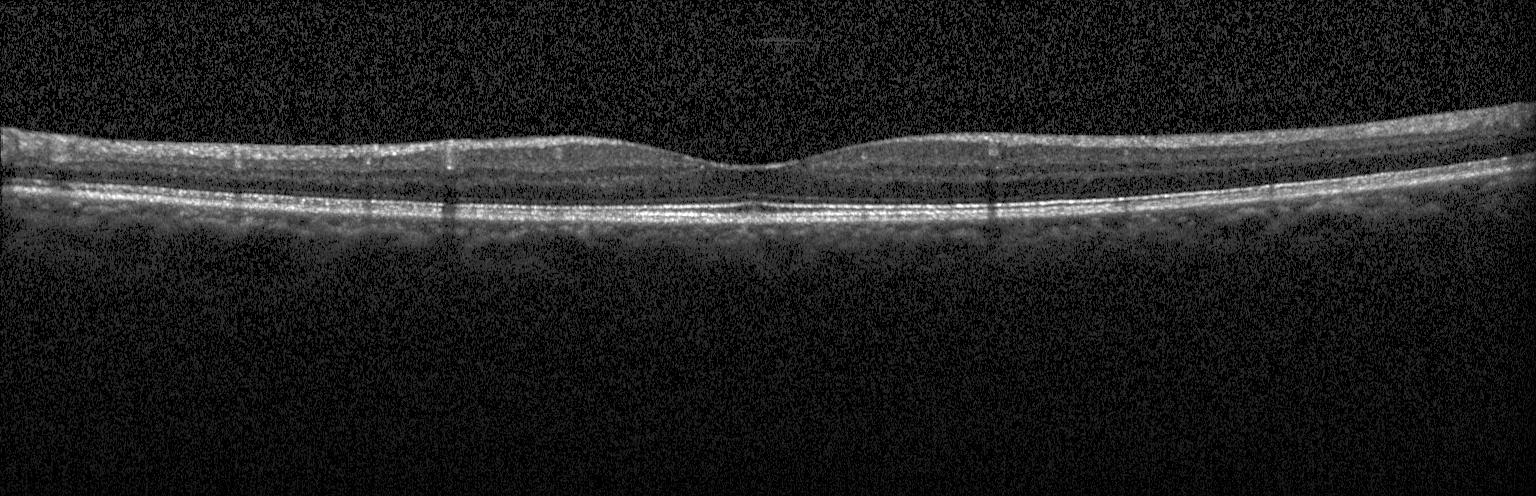 Retinal OCT cross-section · horizontal scan through the fovea · spectral-domain optical coherence tomography · instrument: Heidelberg Spectralis. Finding: no CNV, no DME, and no drusen.